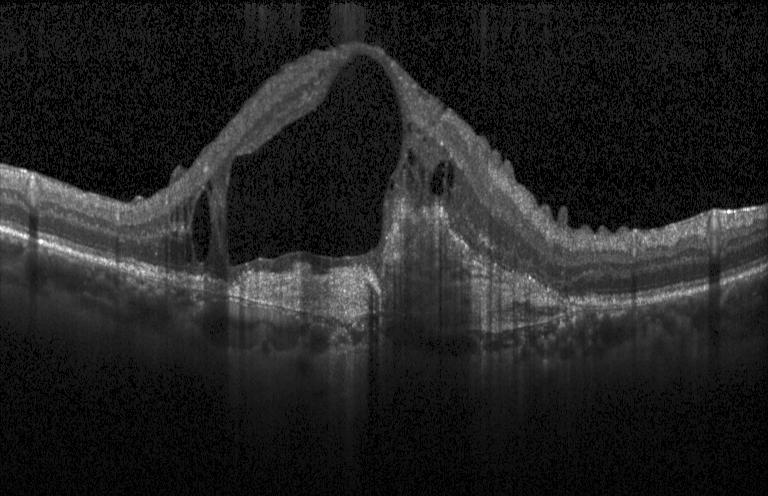
Through the macula; OCT line scan; acquired on a Heidelberg Spectralis — Finding: a choroidal neovascular membrane.